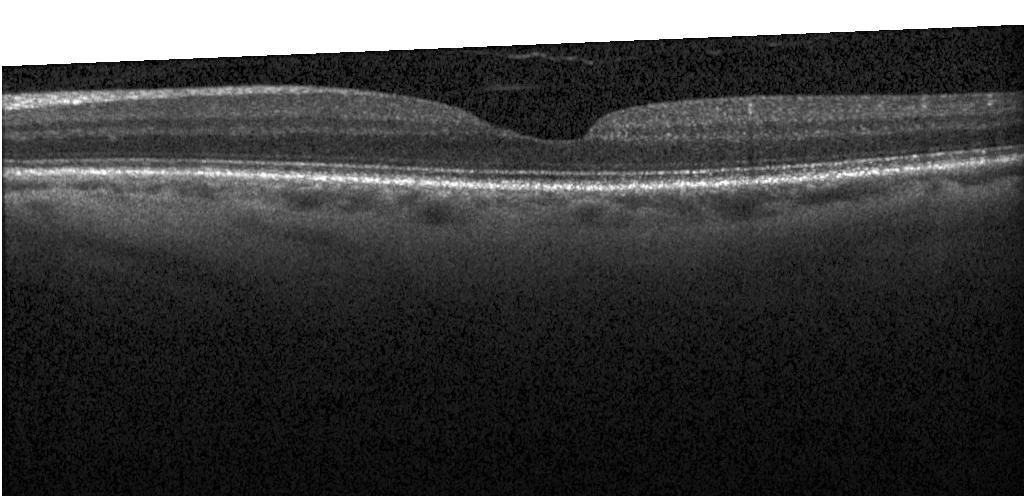
Diagnosis: no evidence of choroidal neovascularization, diabetic macular edema, or drusen.